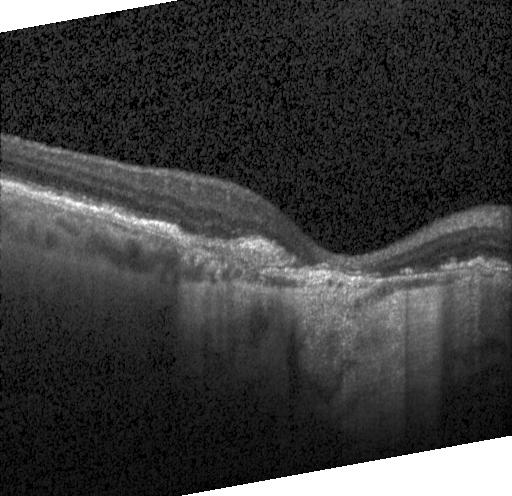 Macular OCT: a choroidal neovascular membrane.